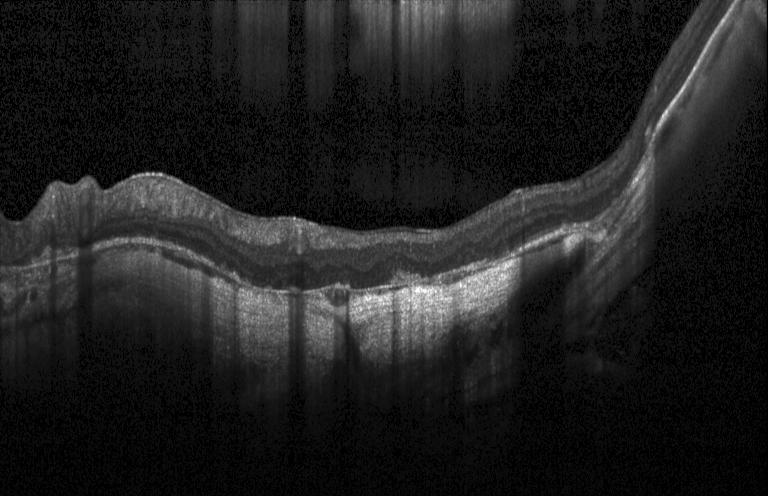 Choroidal neovascularization.